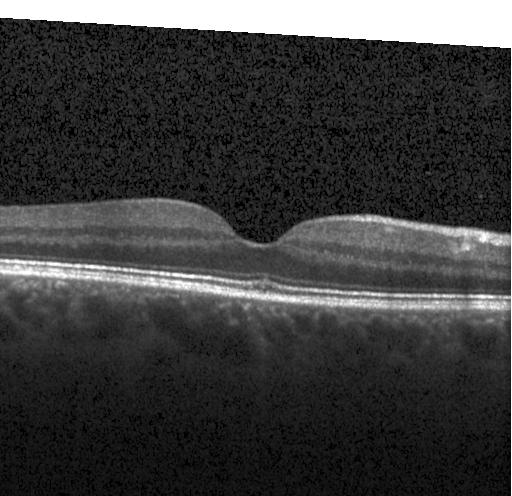
No evidence of choroidal neovascularization, diabetic macular edema, or drusen.